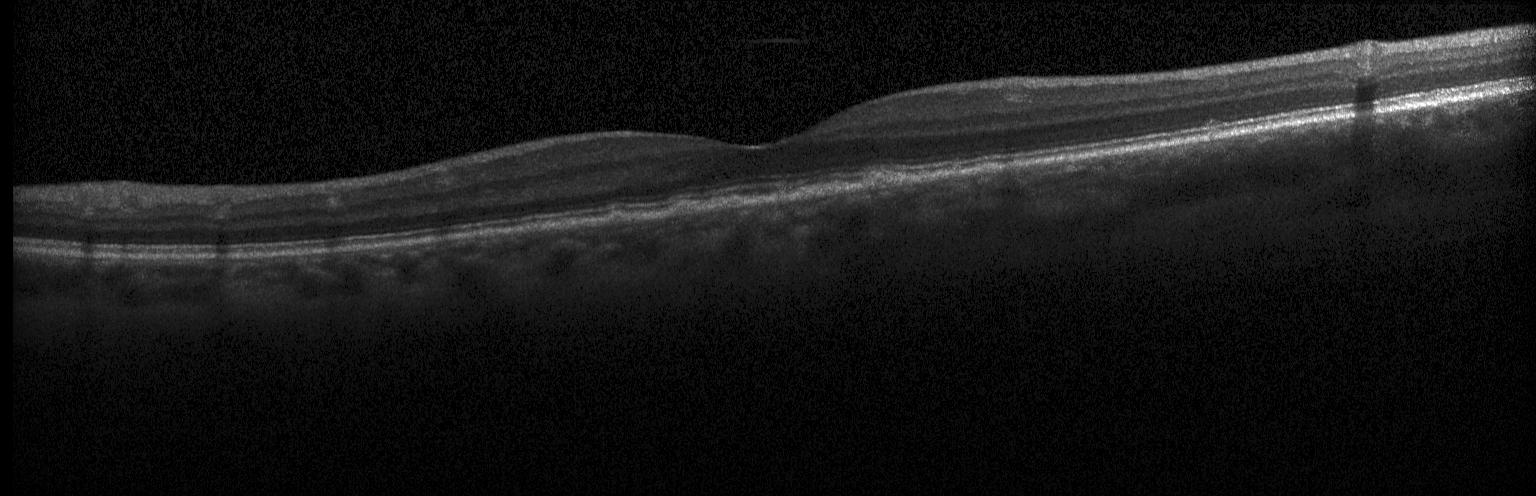
Heidelberg Spectralis. Horizontal scan through the fovea. OCT line scan. Drusen.